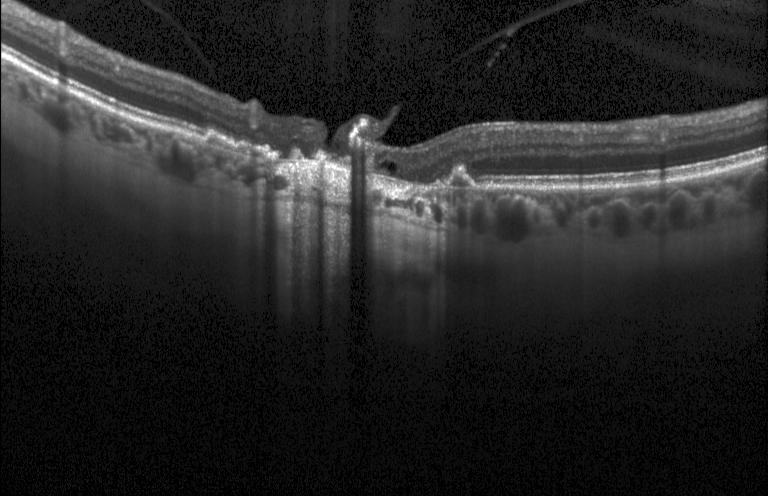
Optical coherence tomography scan. Heidelberg Spectralis OCT system.
Diagnosis: a choroidal neovascular membrane.